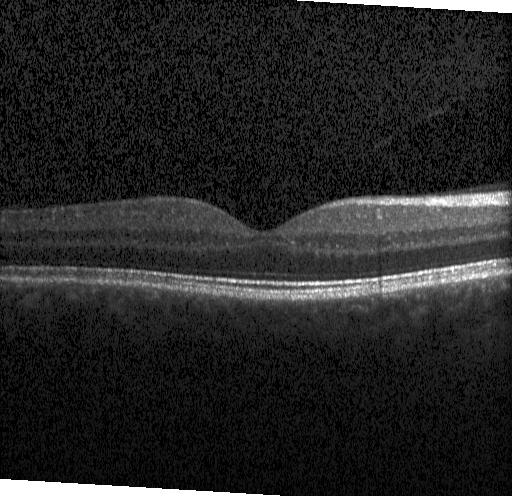

Spectral-domain OCT; instrument: Heidelberg Spectralis; retinal OCT B-scan
The scan shows no evidence of choroidal neovascularization, diabetic macular edema, or drusen.